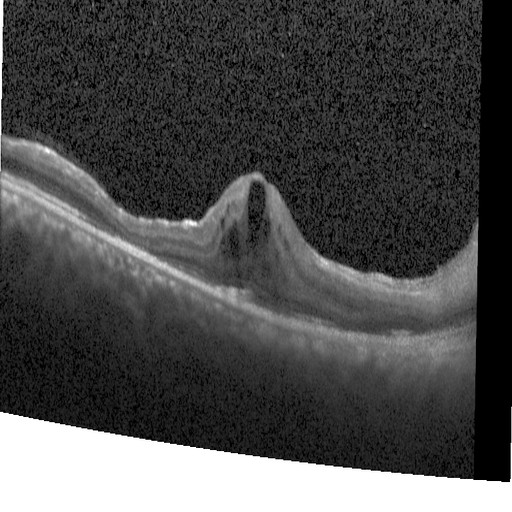

OCT B-scan
Diagnosis: diabetic macular edema.